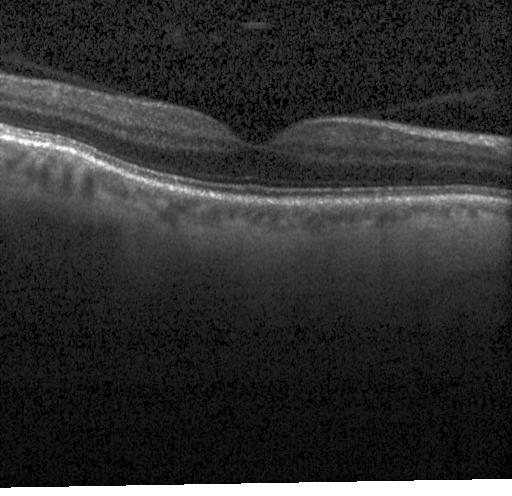

Dx: no choroidal neovascularization, no diabetic macular edema, and no drusen.